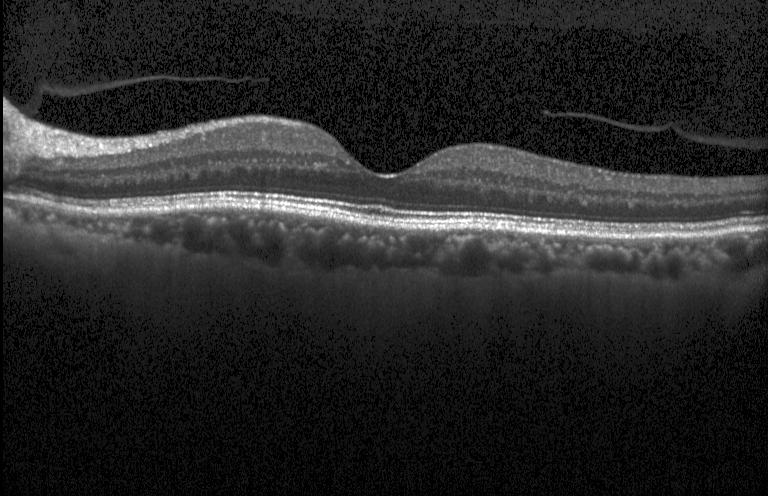

Finding: neither choroidal neovascularization, diabetic macular edema, nor drusen.